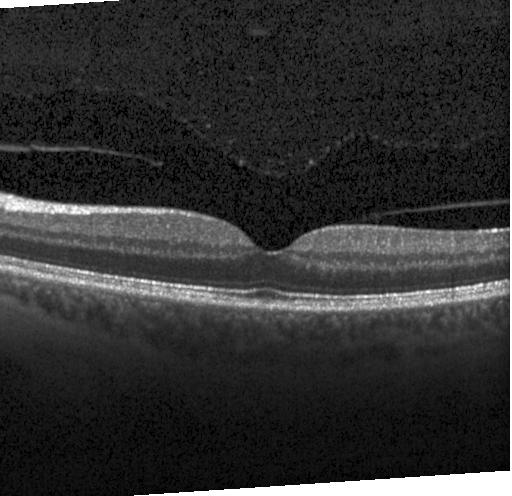 No evidence of choroidal neovascularization, diabetic macular edema, or drusen.